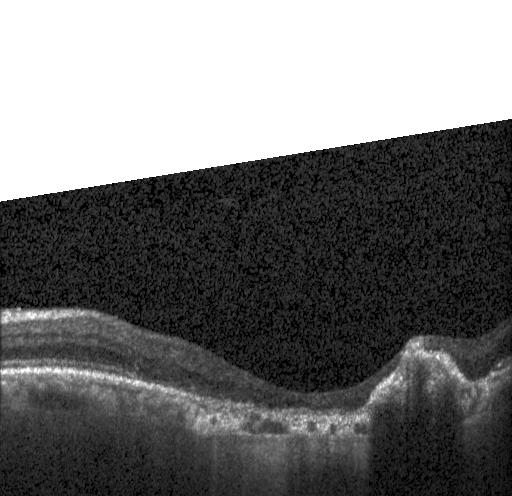 Retinal OCT cross-section showing choroidal neovascularization (CNV).